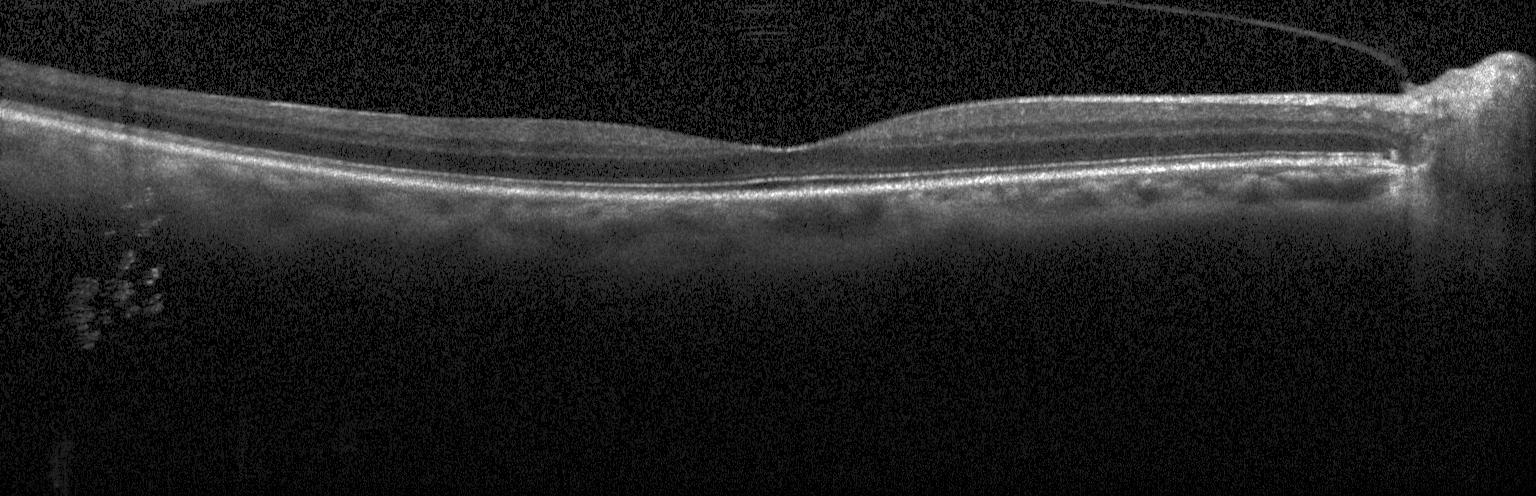

Fovea-centered · SD-OCT · OCT B-scan · acquired on a Heidelberg Spectralis. Finding: no choroidal neovascularization, diabetic macular edema, or drusen.